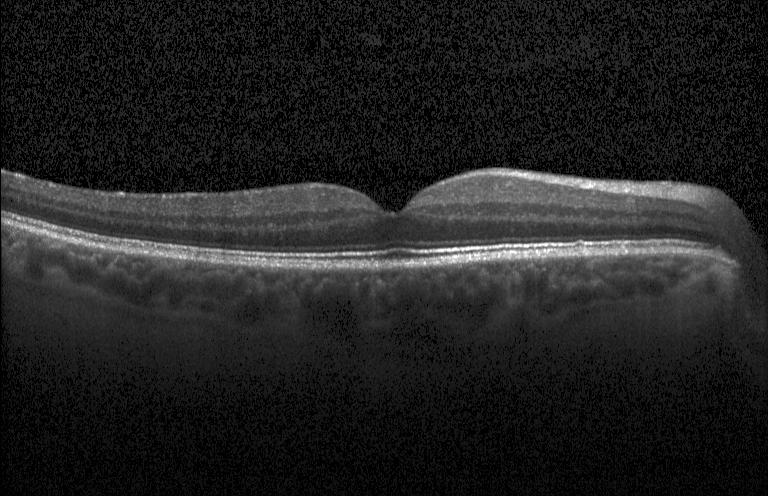 Optical coherence tomography scan
Diagnosis: no choroidal neovascularization, diabetic macular edema, or drusen.